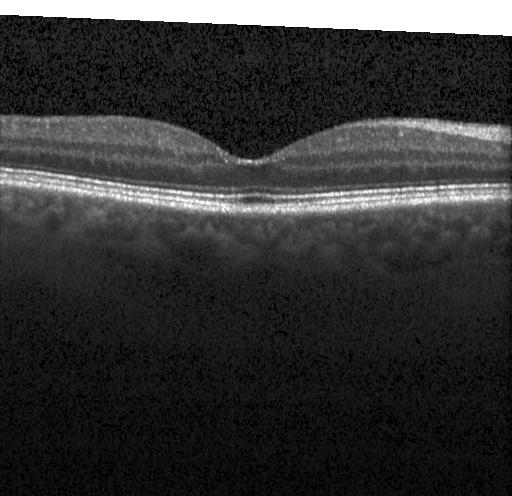
Through the macula. OCT B-scan. Instrument: Heidelberg Spectralis — This B-scan demonstrates no choroidal neovascularization, diabetic macular edema, or drusen.